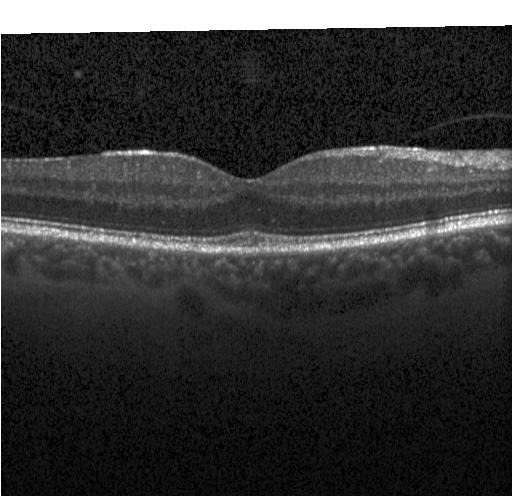
Dx: no evidence of CNV, DME, or drusen.